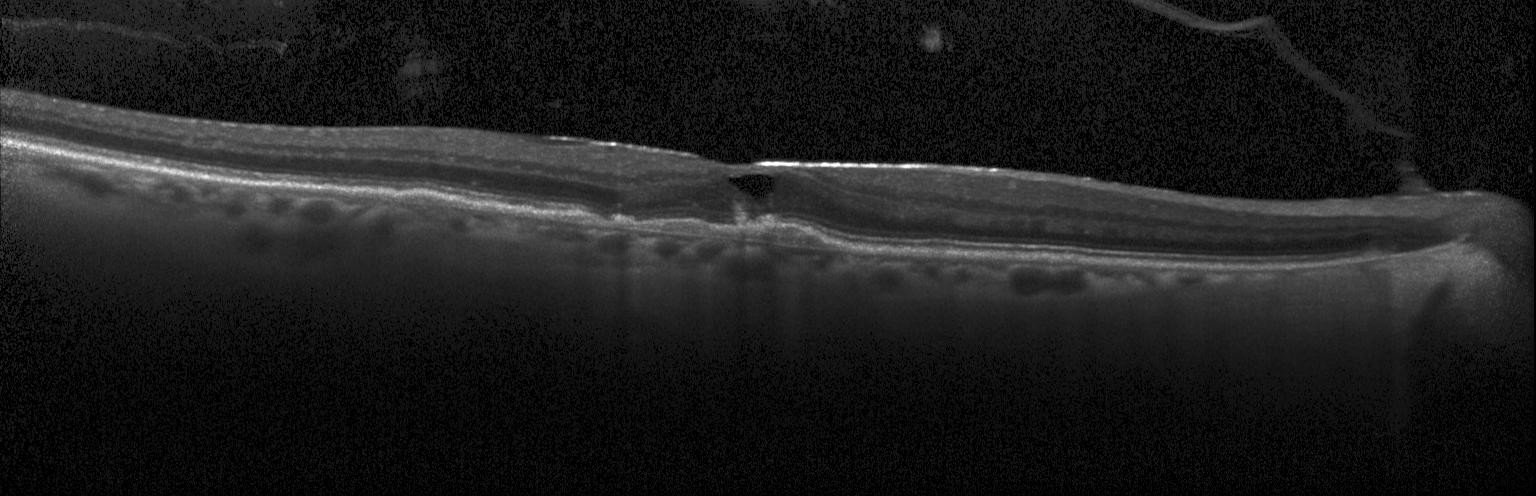
Finding: a choroidal neovascular membrane.